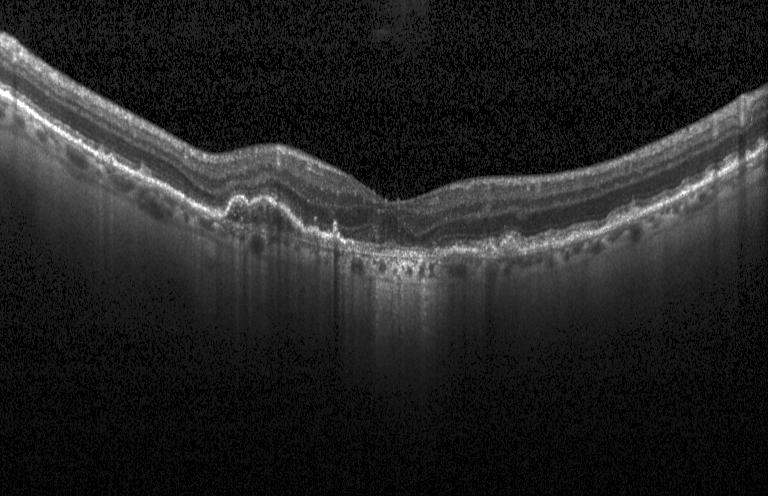

Instrument: Heidelberg Spectralis · centered on the fovea · retinal OCT cross-section
Dx: a choroidal neovascular membrane.